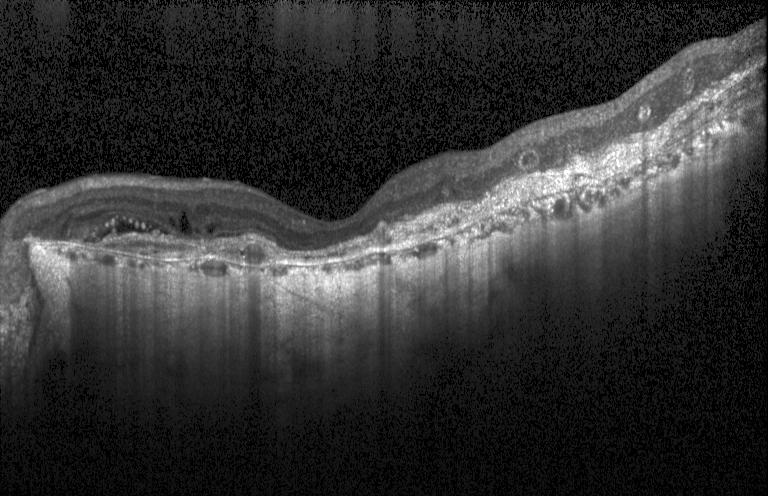 Optical coherence tomography B-scan — OCT finding: a choroidal neovascular membrane.